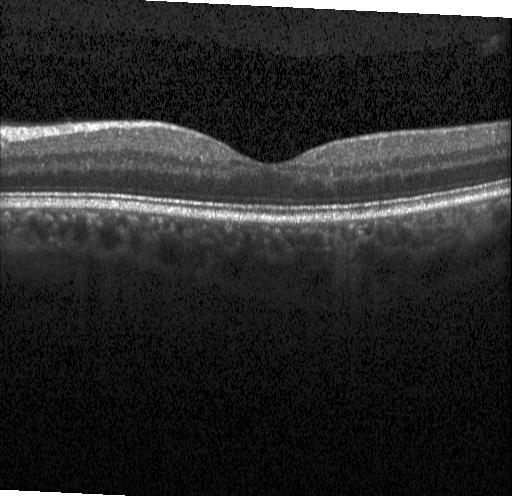 Retinal OCT cross-section · horizontal scan through the fovea. Impression: neither choroidal neovascularization, diabetic macular edema, nor drusen.